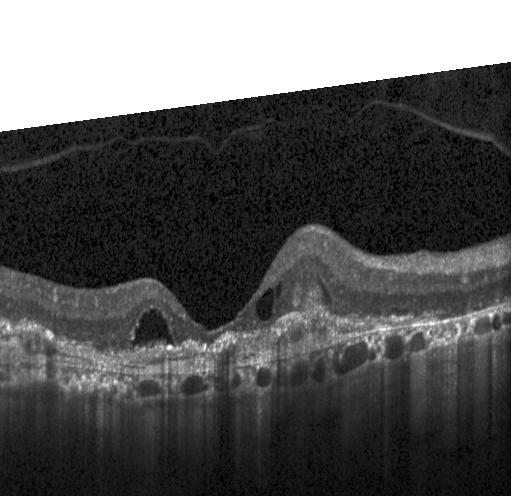 CNV.